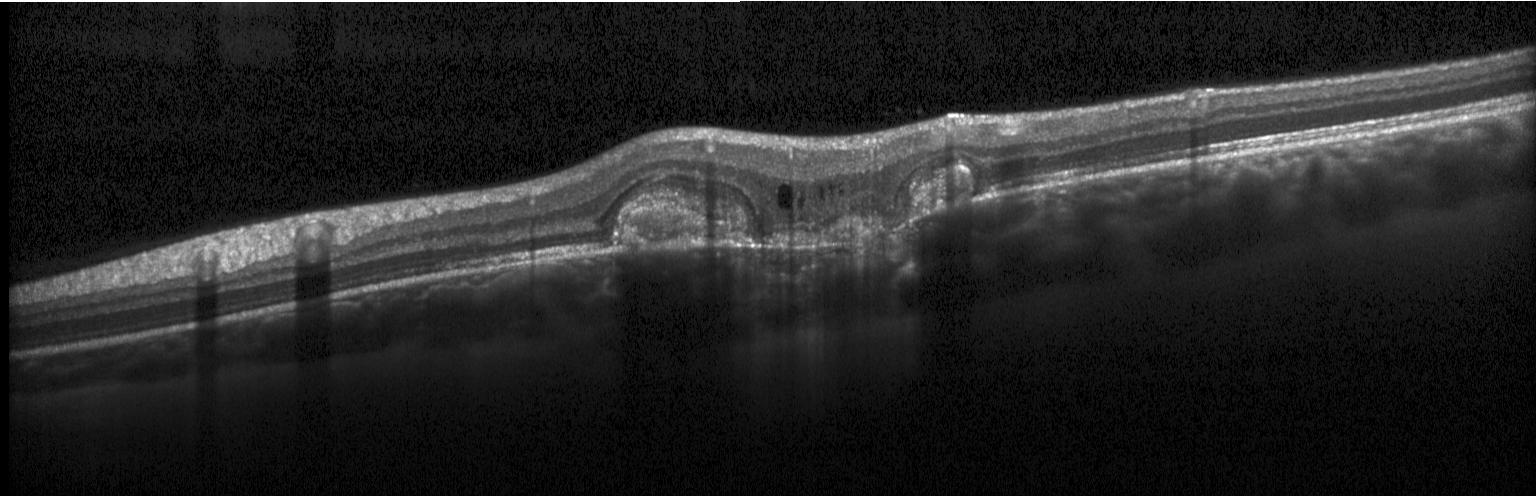
Diagnosis: CNV.